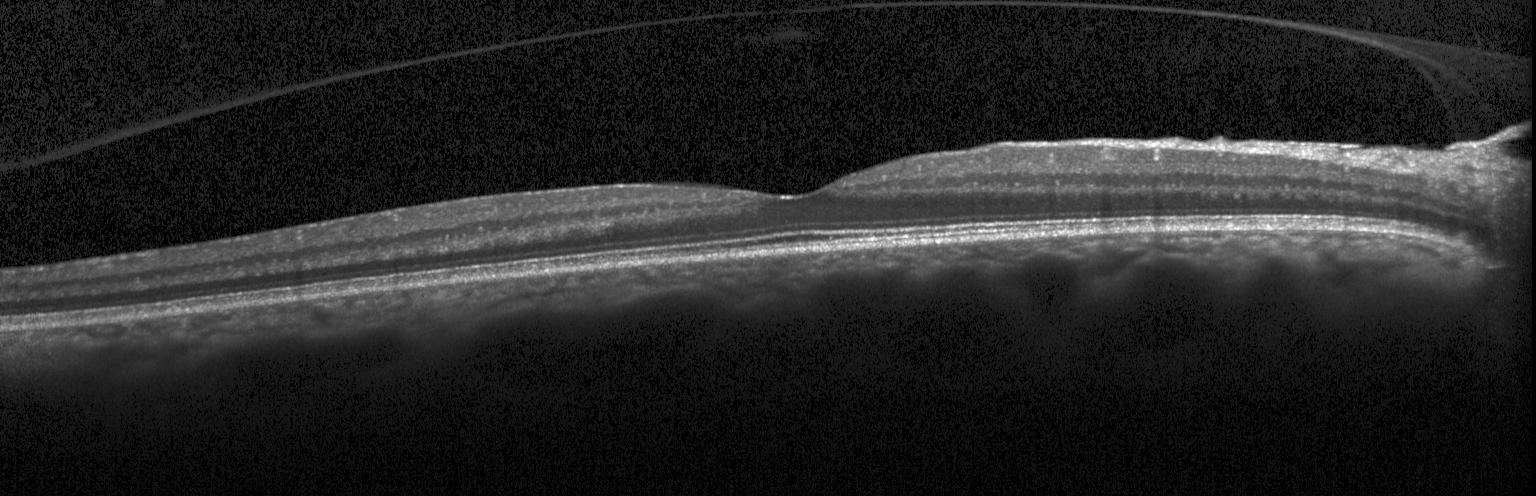 Retinal OCT cross-section. OCT finding: neither CNV, DME, nor drusen.